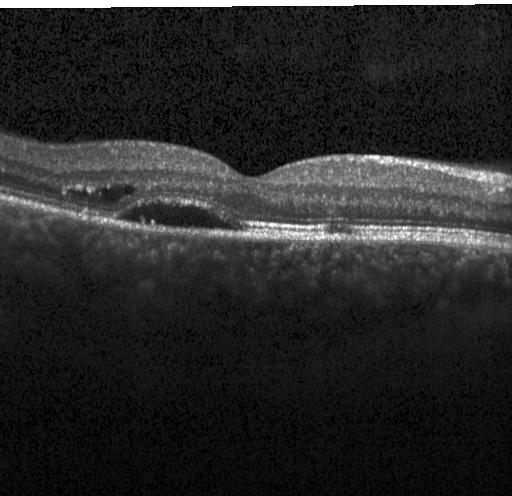

OCT scan showing CNV.